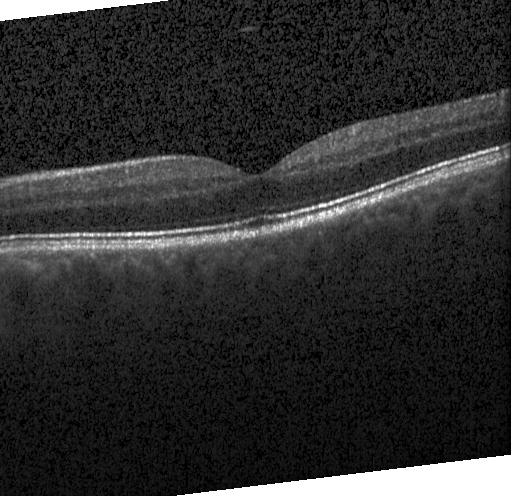
OCT line scan.
Finding: no evidence of choroidal neovascularization, diabetic macular edema, or drusen.